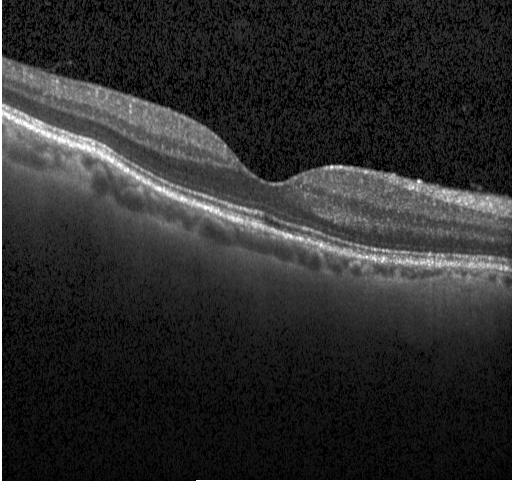
Fovea-centered. Optical coherence tomography B-scan. Heidelberg Spectralis OCT system
This B-scan demonstrates no CNV, DME, or drusen.